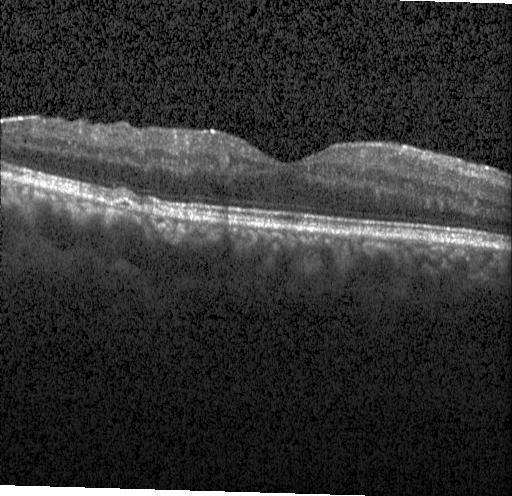

Spectral-domain OCT B-scan: drusen.